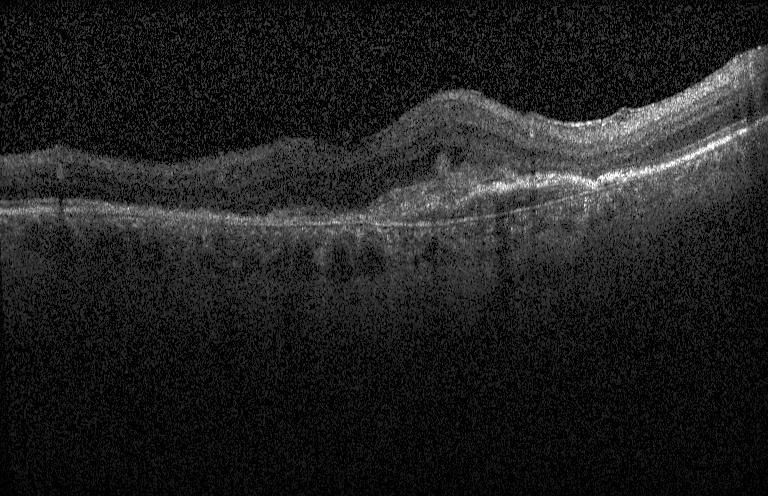

Retinal OCT B-scan, Heidelberg Spectralis — Dx: CNV.